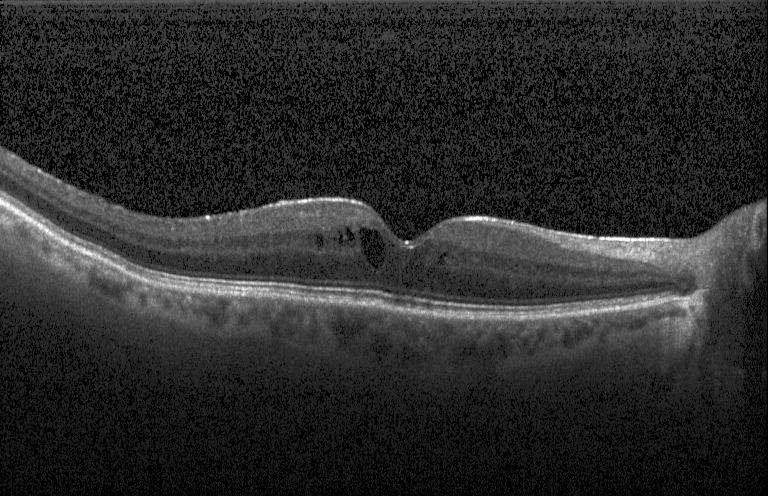 Retinal OCT B-scan · Heidelberg Spectralis OCT system.
Diagnosis: diabetic macular edema.